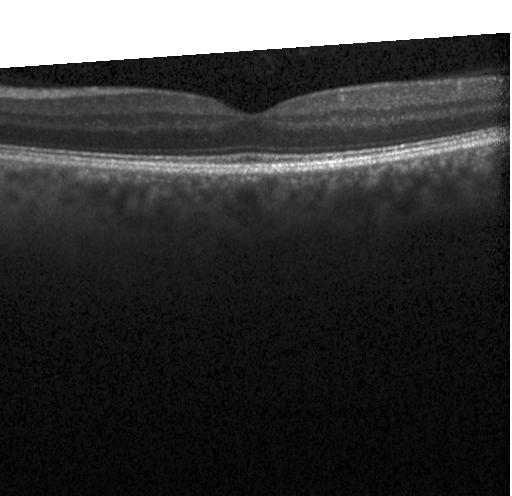

Impression: neither choroidal neovascularization, diabetic macular edema, nor drusen.